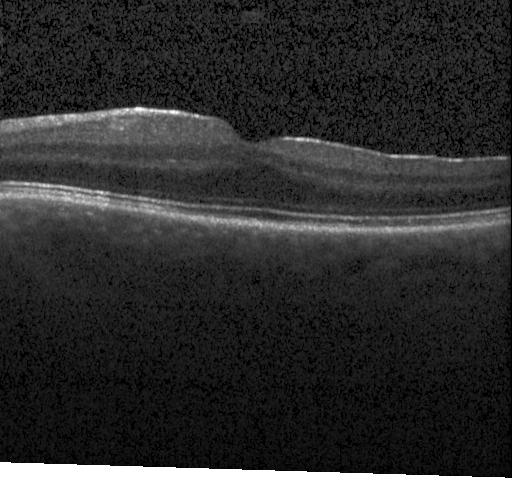
Spectral-domain OCT, retinal OCT B-scan. No CNV, DME, or drusen.